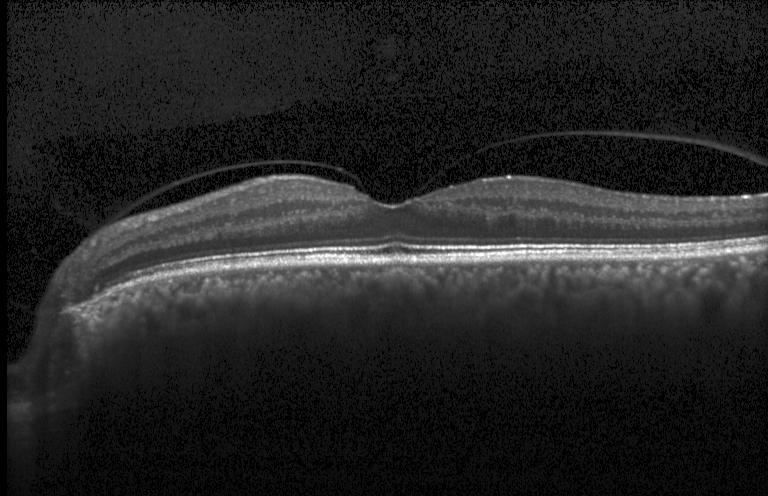

Macular OCT: no evidence of choroidal neovascularization, diabetic macular edema, or drusen.